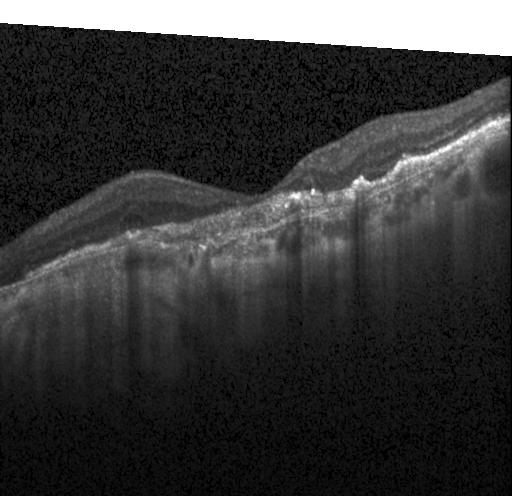 OCT scan showing a choroidal neovascular membrane.